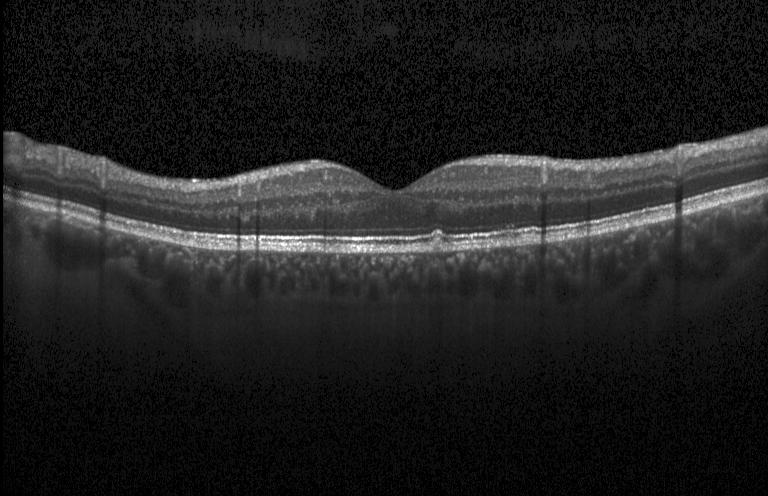

Spectral-domain optical coherence tomography · optical coherence tomography B-scan · Heidelberg Spectralis OCT system · through the macula. The scan shows drusen.